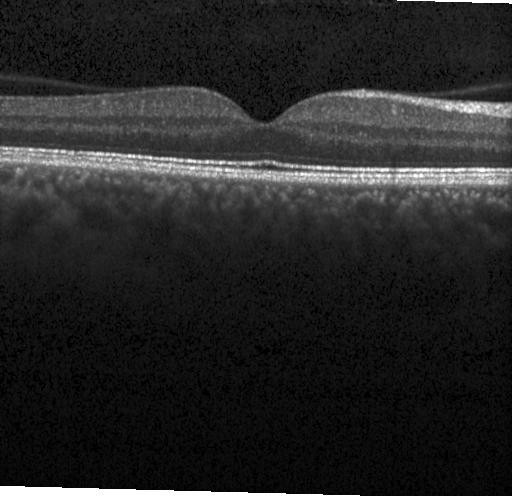

Impression: no choroidal neovascularization, diabetic macular edema, or drusen.